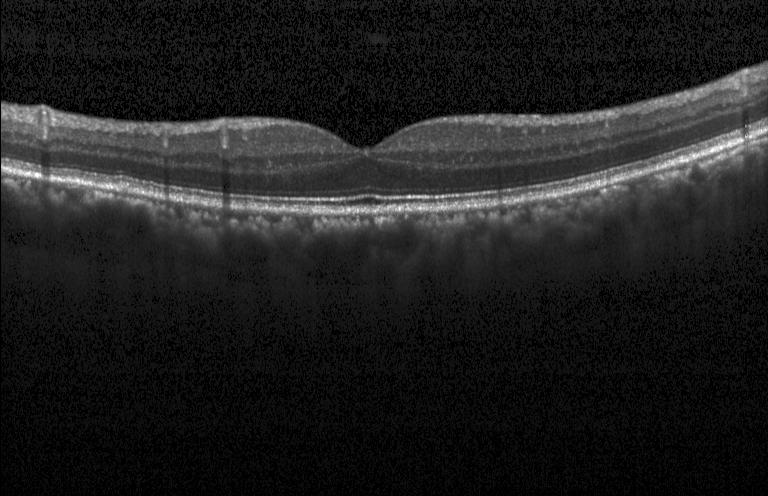 Finding: no evidence of choroidal neovascularization, diabetic macular edema, or drusen.